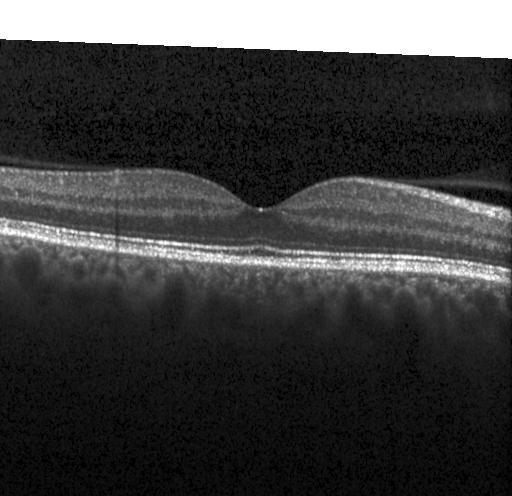
OCT line scan; spectral-domain OCT — This B-scan demonstrates neither CNV, DME, nor drusen.